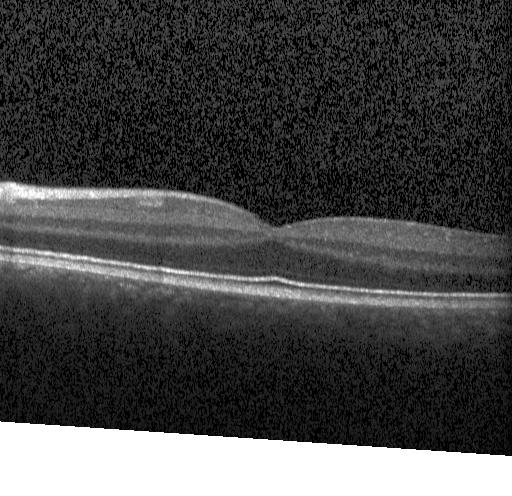 Instrument: Heidelberg Spectralis, optical coherence tomography B-scan
The scan shows neither choroidal neovascularization, diabetic macular edema, nor drusen.